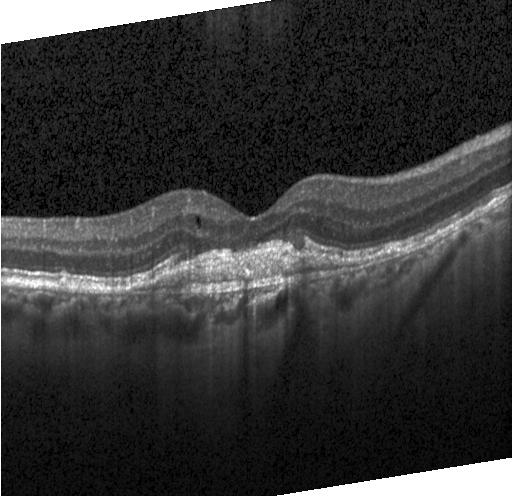
The scan shows CNV.